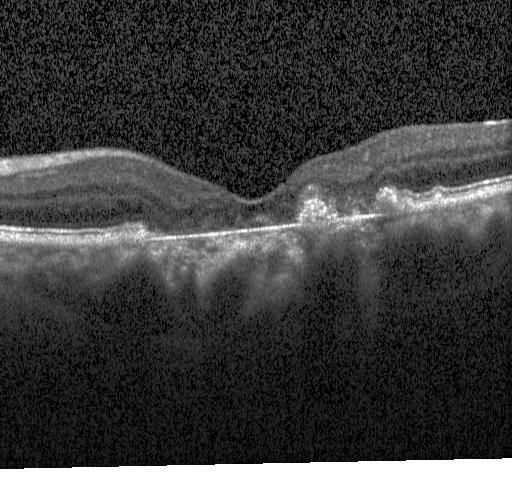 Retinal OCT cross-section. SD-OCT. Macular scan
Dx: choroidal neovascularization.